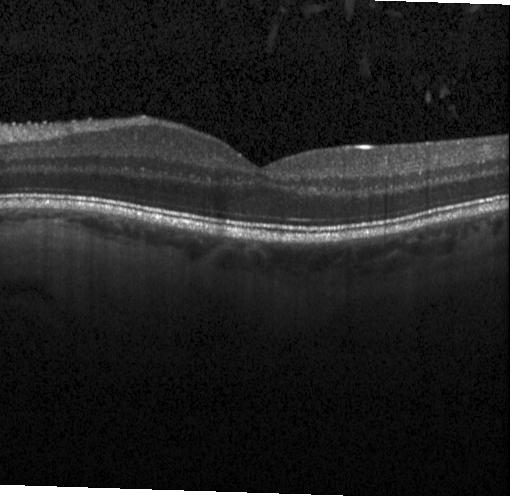
Fovea-centered · optical coherence tomography B-scan
Impression: no CNV, DME, or drusen.